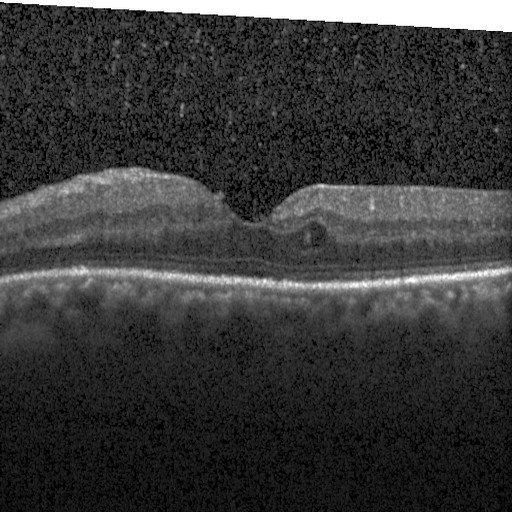

OCT line scan.
Impression: diabetic macular edema.